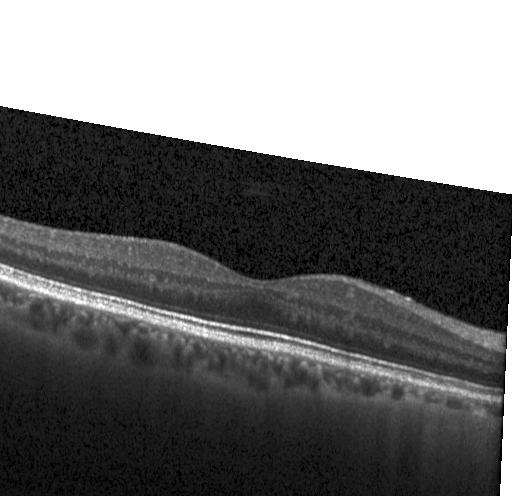
SD-OCT. Optical coherence tomography scan. Heidelberg Spectralis OCT system
Diagnosis: no choroidal neovascularization, diabetic macular edema, or drusen.